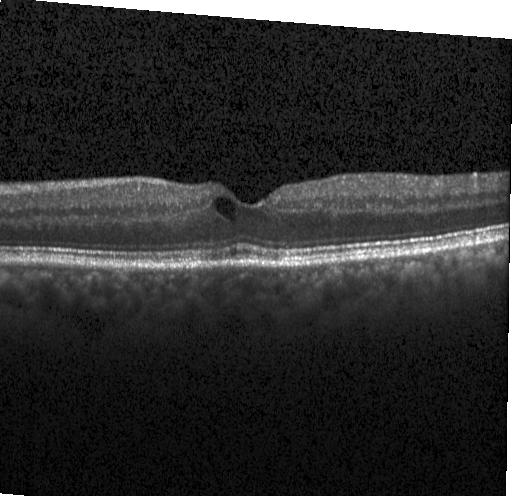

SD-OCT, horizontal scan through the fovea, OCT B-scan, instrument: Heidelberg Spectralis — Macular OCT: DME.